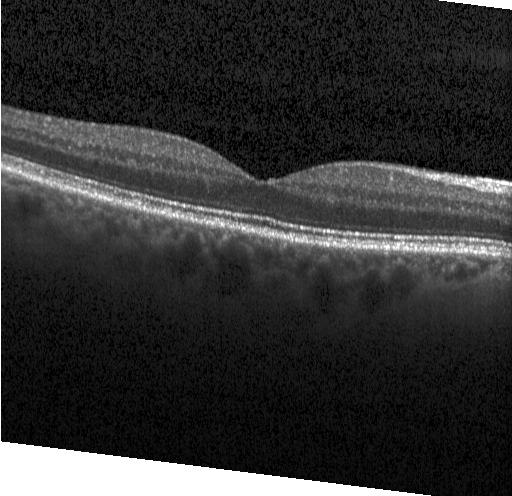
Spectral-domain OCT · Heidelberg Spectralis · horizontal scan through the fovea · optical coherence tomography scan. Finding: no CNV, no DME, and no drusen.